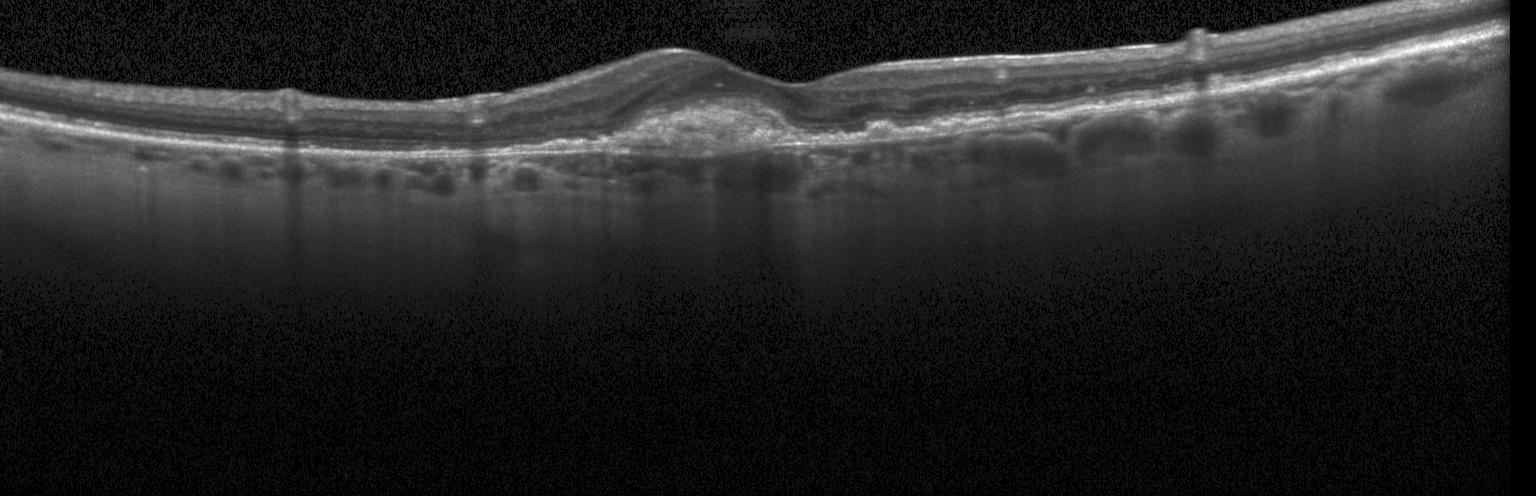

OCT finding: CNV.